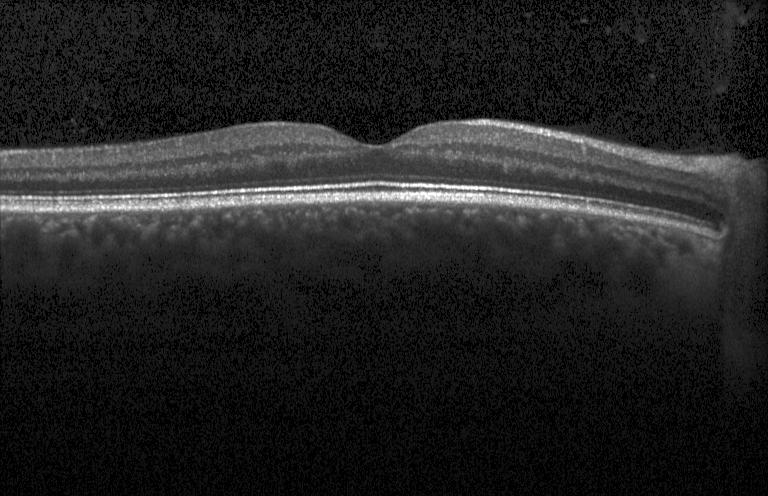
Macular OCT: no evidence of choroidal neovascularization, diabetic macular edema, or drusen.